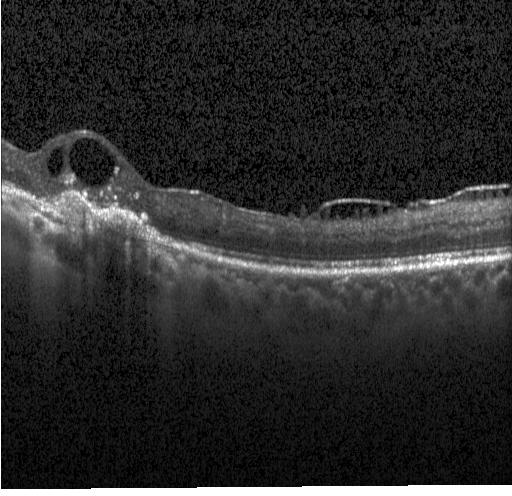
Optical coherence tomography scan.
Choroidal neovascularization.